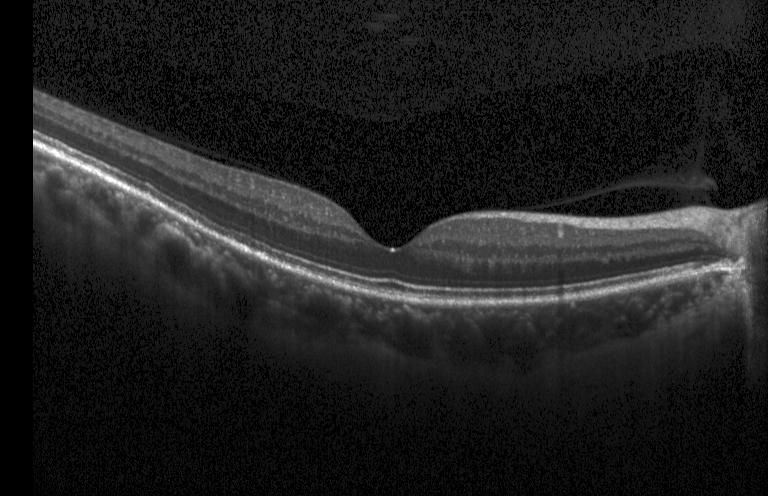
Diagnosis: no choroidal neovascularization, diabetic macular edema, or drusen.